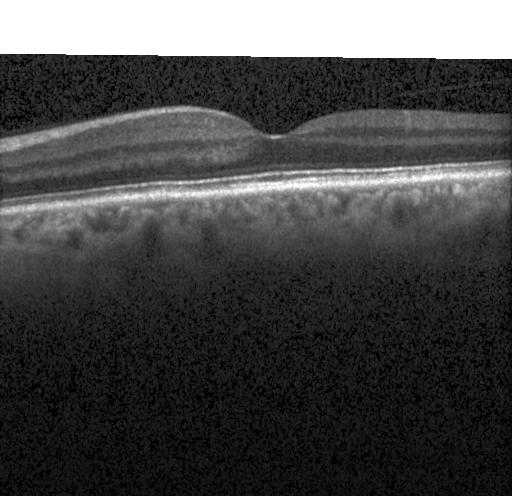 Through the macula; Heidelberg Spectralis OCT system; optical coherence tomography scan; SD-OCT
Impression: no evidence of choroidal neovascularization, diabetic macular edema, or drusen.